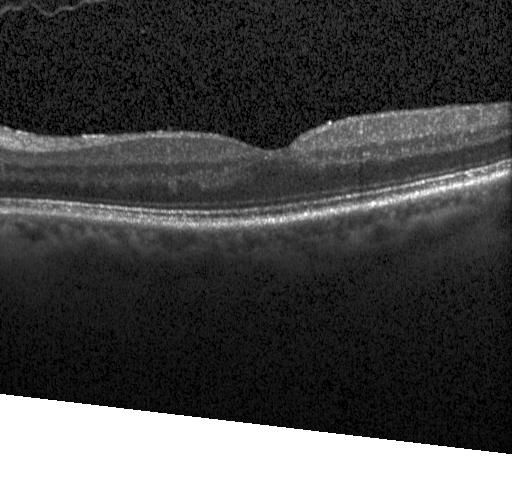 OCT scan showing no evidence of choroidal neovascularization, diabetic macular edema, or drusen.